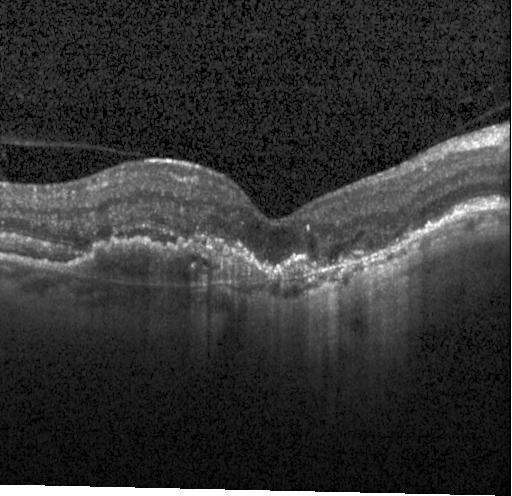
Instrument: Heidelberg Spectralis, optical coherence tomography B-scan, spectral-domain OCT, through the macula. Impression: a choroidal neovascular membrane.